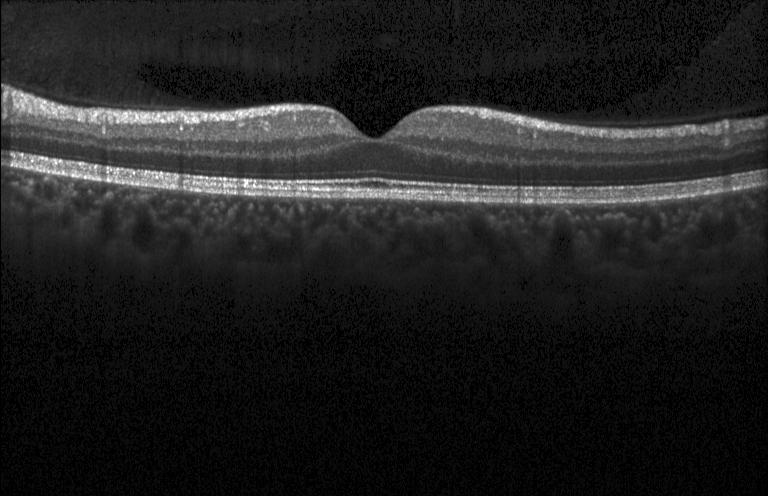

Dx: no evidence of CNV, DME, or drusen.